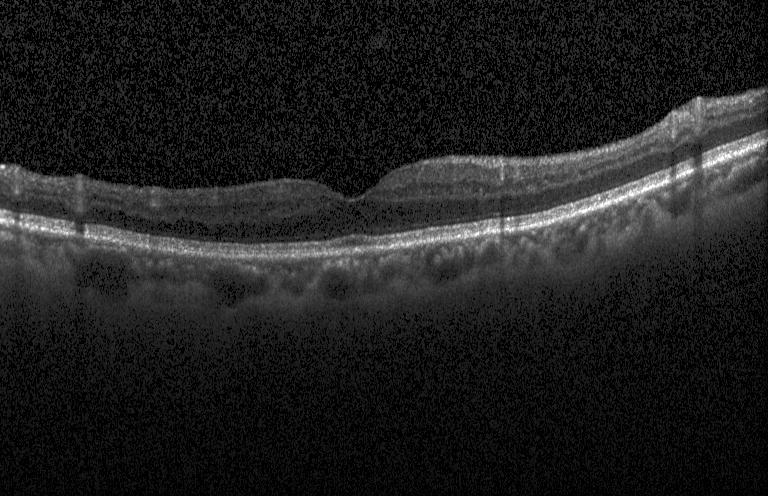
Heidelberg Spectralis. Horizontal scan through the fovea. OCT B-scan. Spectral-domain OCT.
The scan shows no evidence of choroidal neovascularization, diabetic macular edema, or drusen.